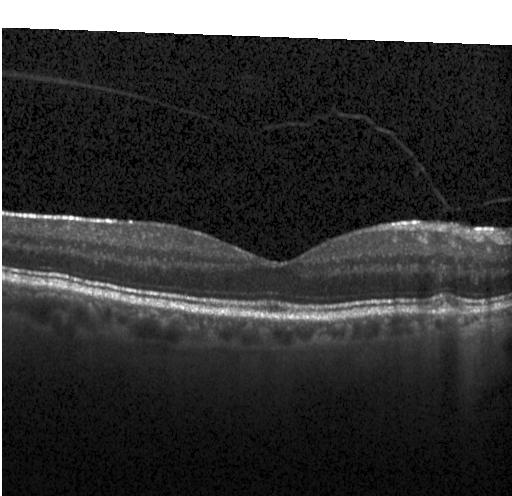
Centered on the fovea. SD-OCT. Optical coherence tomography B-scan. Heidelberg Spectralis. Dx: sub-RPE drusenoid deposits.